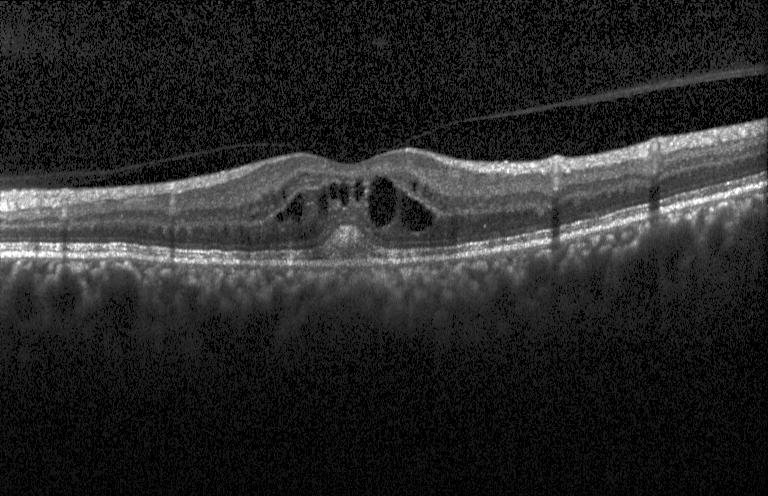

Optical coherence tomography scan. Diagnosis: choroidal neovascularization.